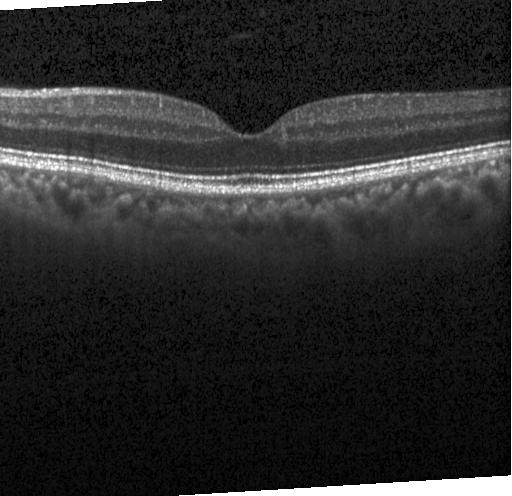

Diagnosis: no evidence of CNV, DME, or drusen.